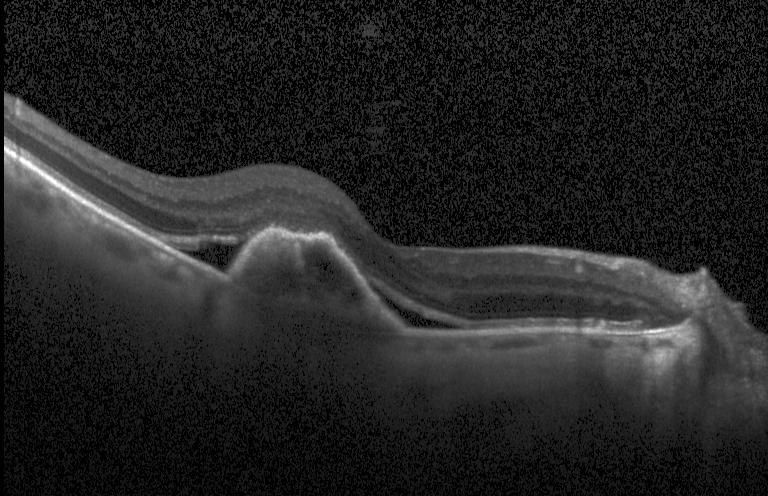
The scan shows choroidal neovascularization.